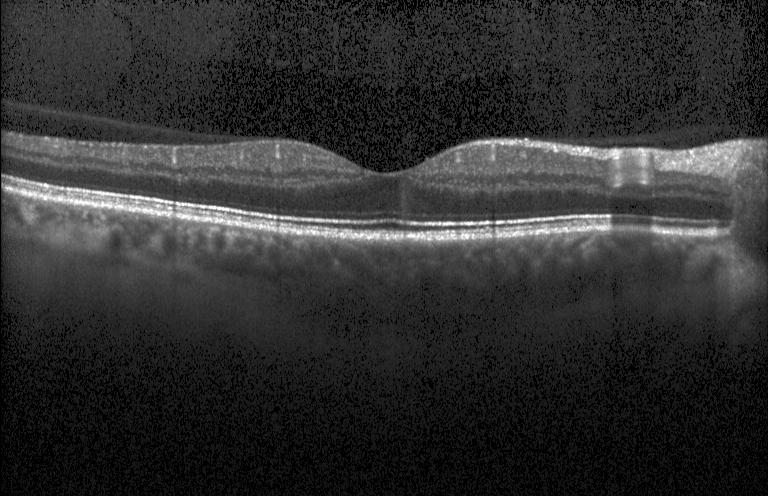

Retinal OCT B-scan; spectral-domain optical coherence tomography.
Diagnosis: neither CNV, DME, nor drusen.